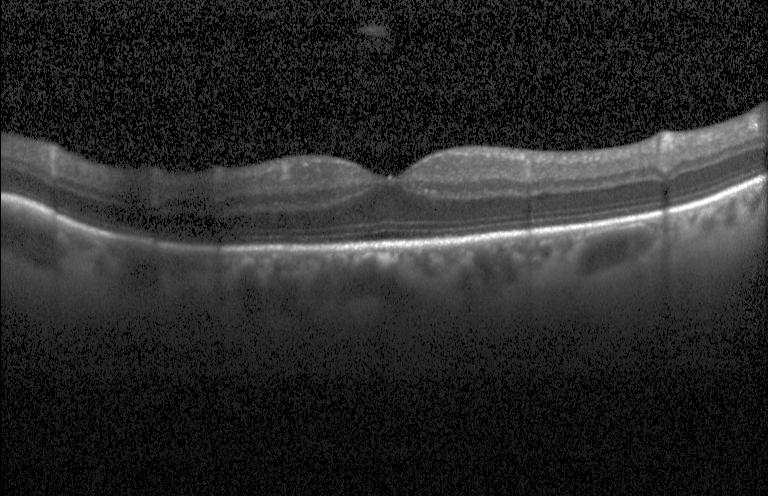

This B-scan demonstrates no evidence of choroidal neovascularization, diabetic macular edema, or drusen.